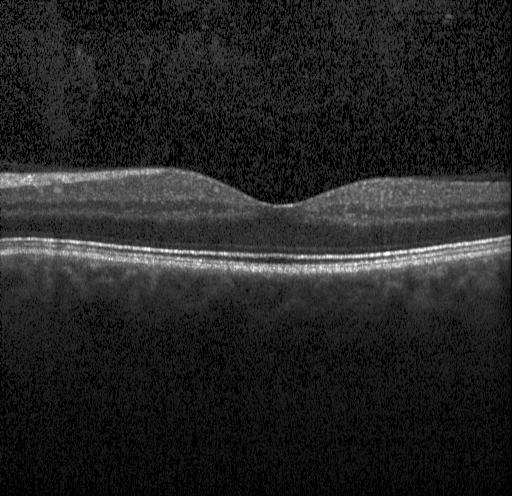
OCT B-scan showing no choroidal neovascularization, no diabetic macular edema, and no drusen.